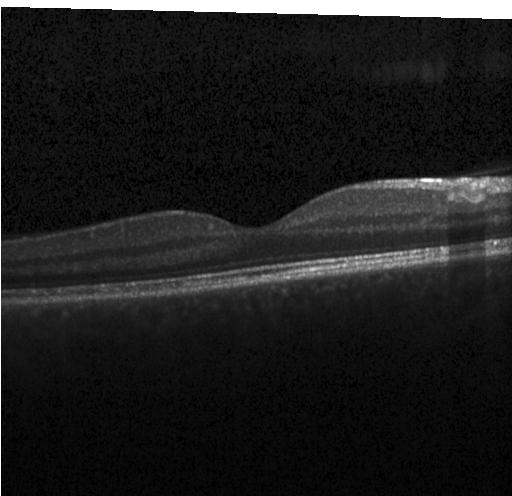
OCT B-scan. Macular scan. Spectral-domain OCT. Instrument: Heidelberg Spectralis. No evidence of CNV, DME, or drusen.